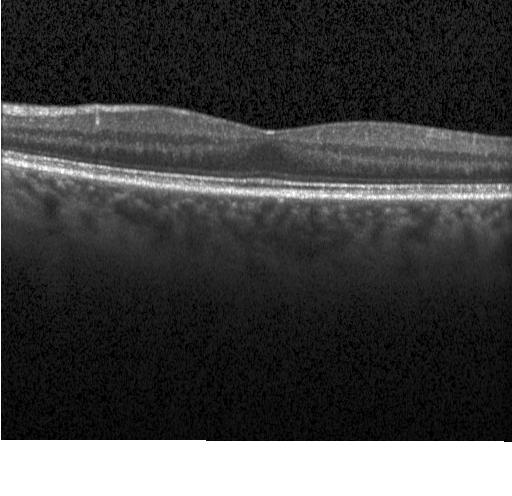
Diagnosis: neither CNV, DME, nor drusen.